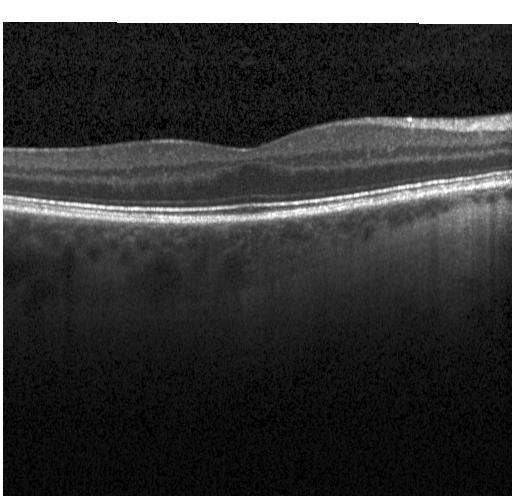 Retinal OCT cross-section.
OCT finding: no CNV, DME, or drusen.